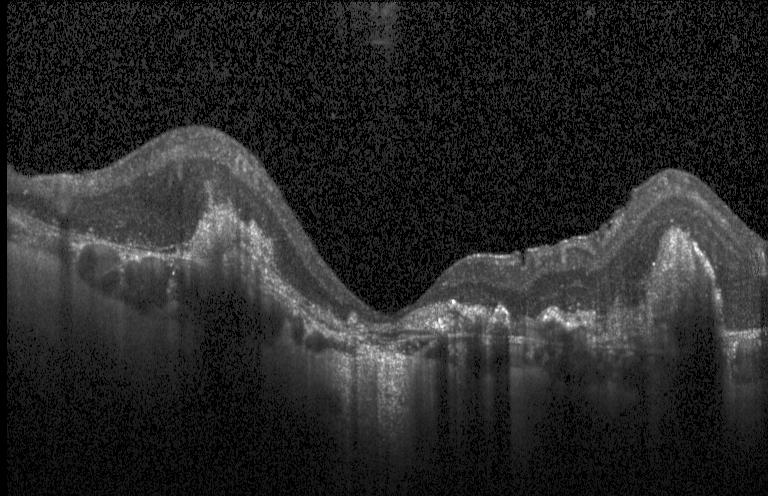

Retinal OCT B-scan.
Impression: a choroidal neovascular membrane.